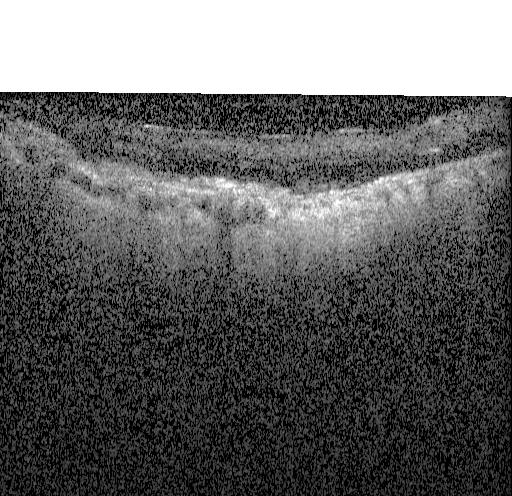
Spectral-domain optical coherence tomography · macular scan · OCT B-scan.
The scan shows a choroidal neovascular membrane.